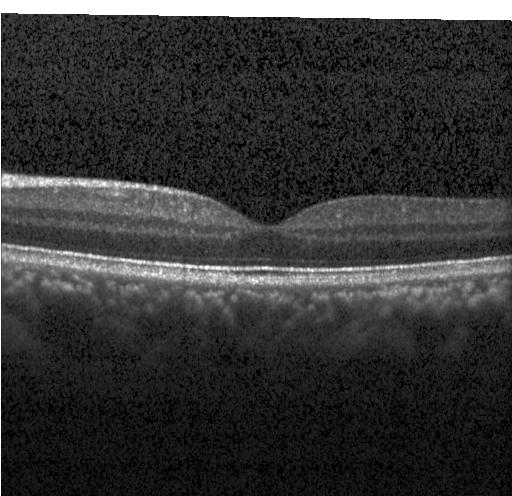
Macular OCT demonstrating no choroidal neovascularization, no diabetic macular edema, and no drusen.